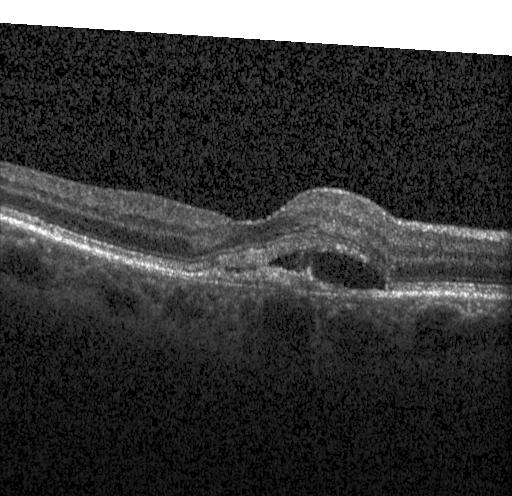

Horizontal scan through the fovea, optical coherence tomography B-scan
Diagnosis: choroidal neovascularization (CNV).